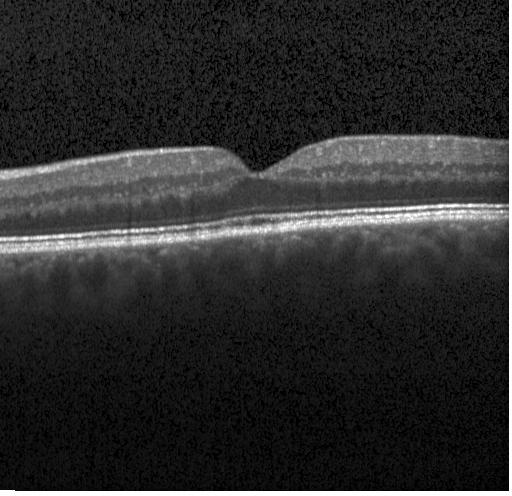

Spectral-domain optical coherence tomography. OCT B-scan. Instrument: Heidelberg Spectralis.
No CNV, DME, or drusen.